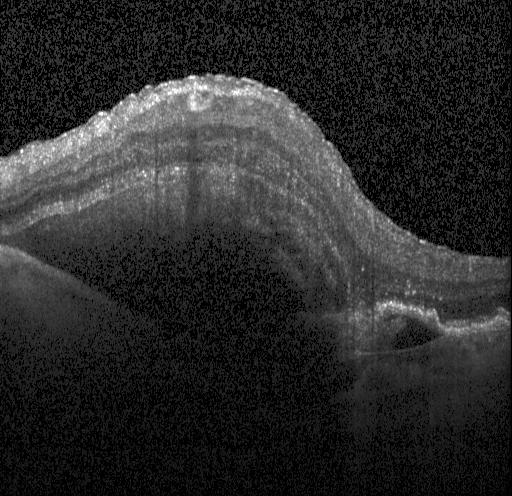 Finding: choroidal neovascularization.